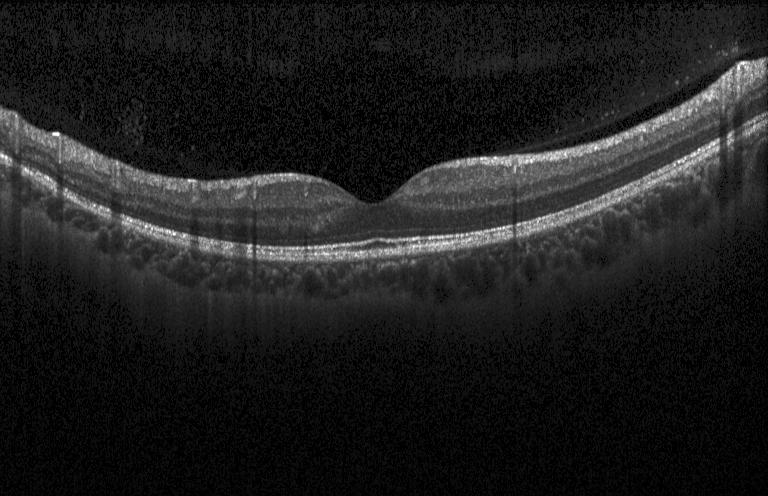

OCT scan showing no choroidal neovascularization, no diabetic macular edema, and no drusen.